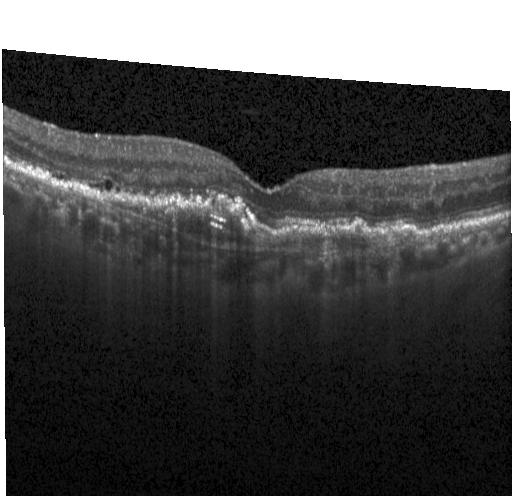 Optical coherence tomography B-scan · instrument: Heidelberg Spectralis · through the macula. Choroidal neovascularization.